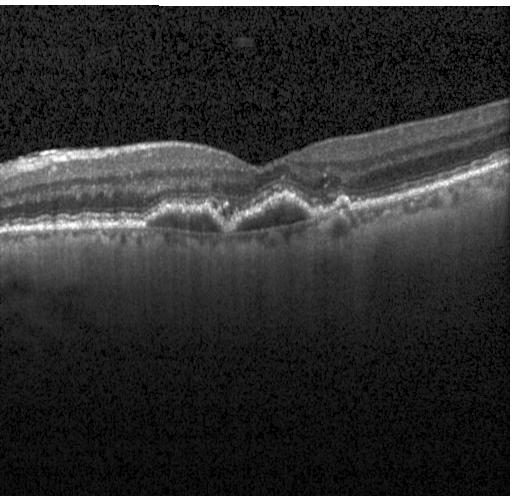
Spectral-domain OCT B-scan: a choroidal neovascular membrane.